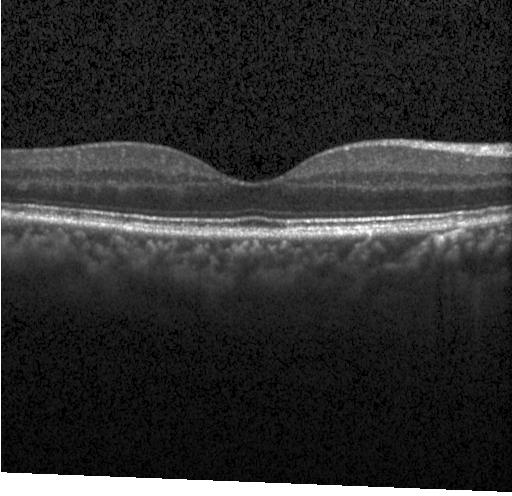
Diagnosis: no choroidal neovascularization, diabetic macular edema, or drusen.